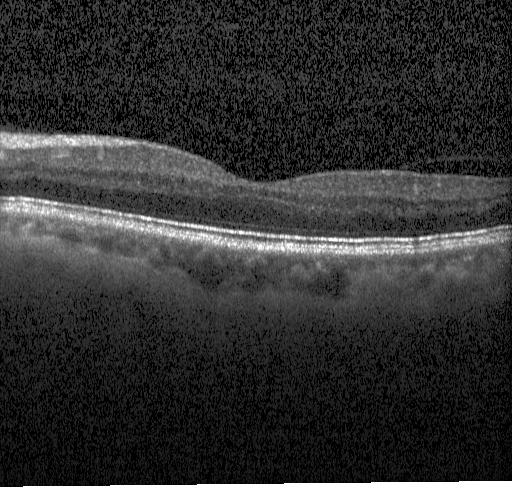 OCT B-scan. Spectral-domain OCT. Heidelberg Spectralis OCT system. This B-scan demonstrates no evidence of choroidal neovascularization, diabetic macular edema, or drusen.